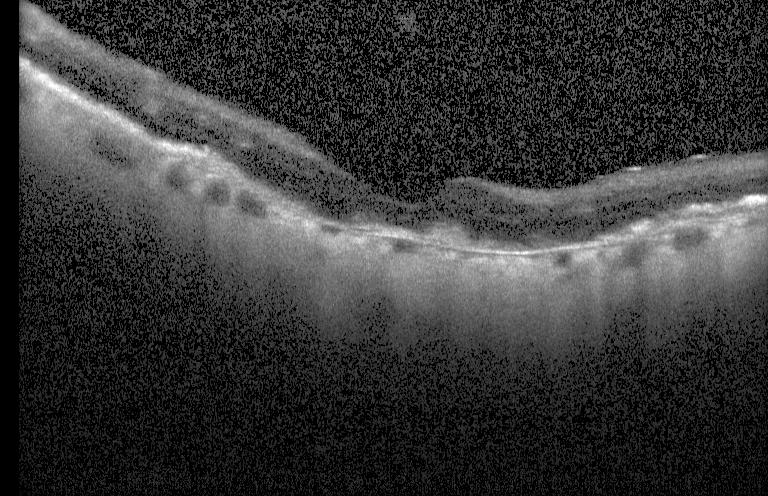 Heidelberg Spectralis OCT system · SD-OCT · optical coherence tomography B-scan · centered on the fovea.
Finding: choroidal neovascularization (CNV).